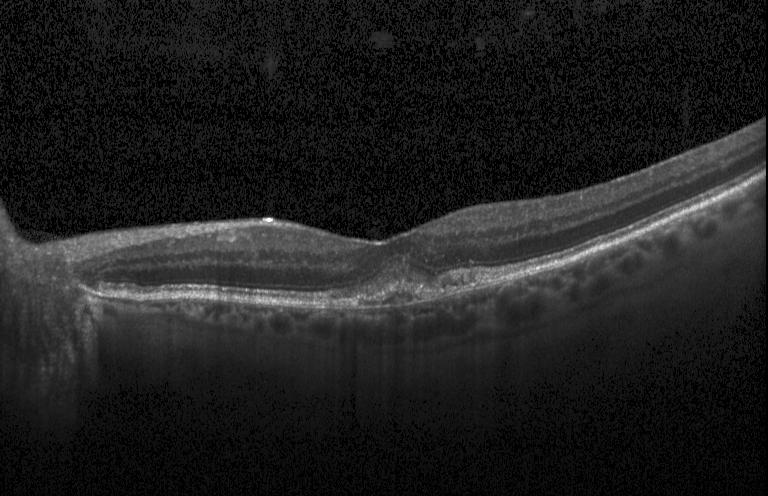

Spectral-domain optical coherence tomography, instrument: Heidelberg Spectralis, centered on the fovea, optical coherence tomography B-scan — The scan shows choroidal neovascularization.